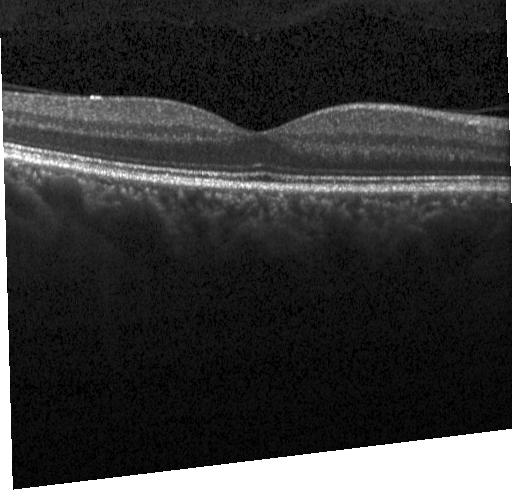

Fovea-centered, Heidelberg Spectralis, spectral-domain optical coherence tomography, optical coherence tomography B-scan
Impression: neither choroidal neovascularization, diabetic macular edema, nor drusen.